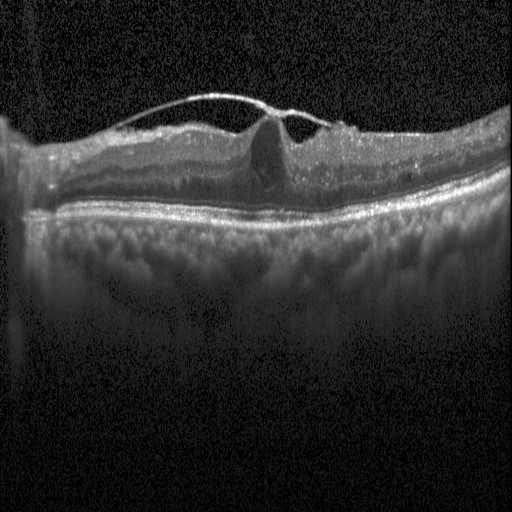

Spectral-domain OCT. Optical coherence tomography B-scan.
OCT finding: DME.